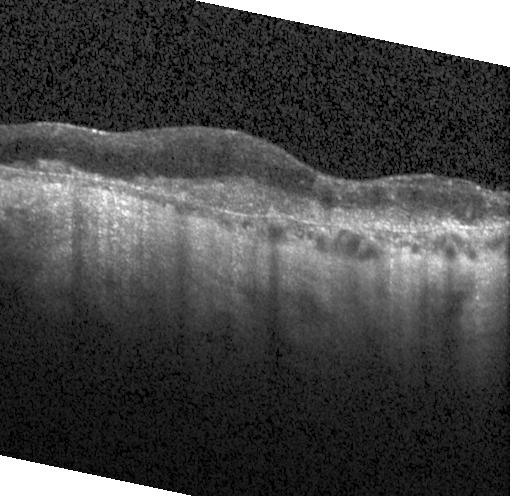

Retinal OCT B-scan — Dx: choroidal neovascularization (CNV).